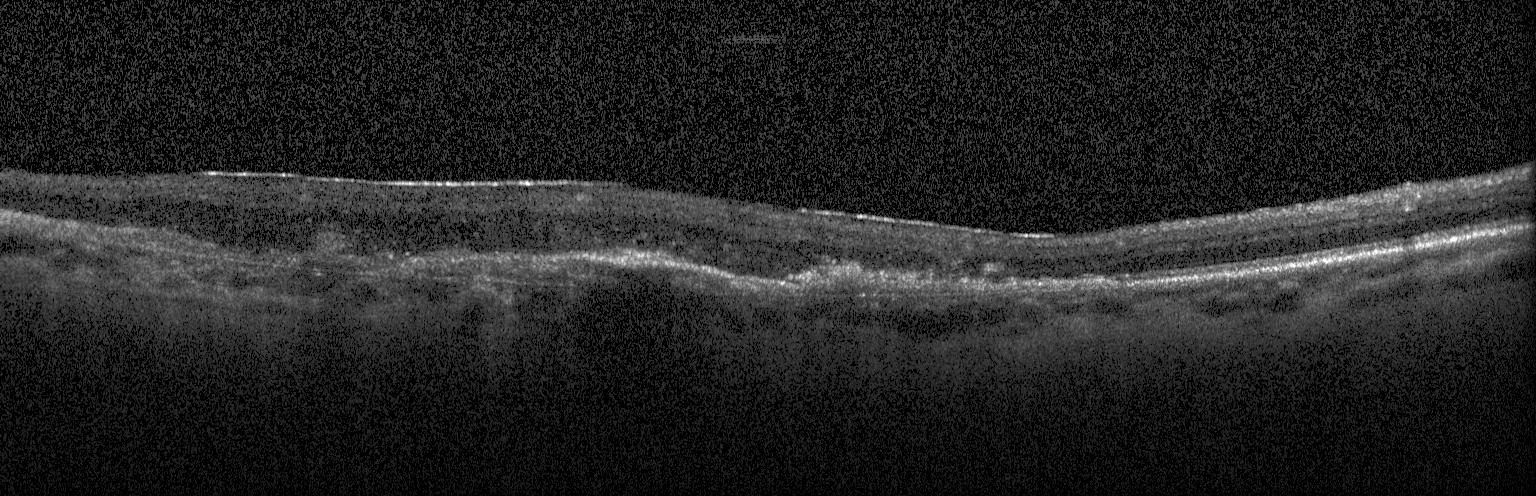 Optical coherence tomography B-scan
Impression: CNV.